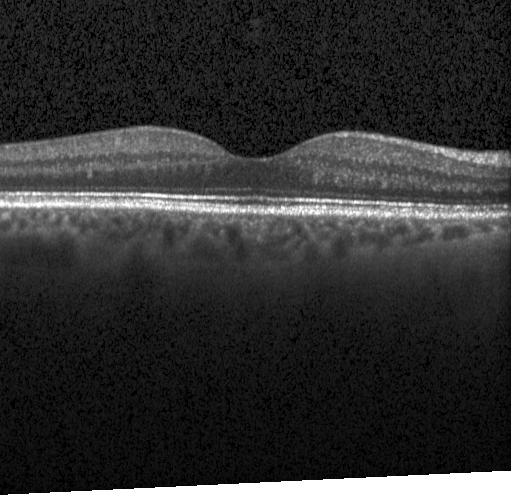 Acquired on a Heidelberg Spectralis · OCT B-scan · SD-OCT · macular scan. Impression: no CNV, DME, or drusen.